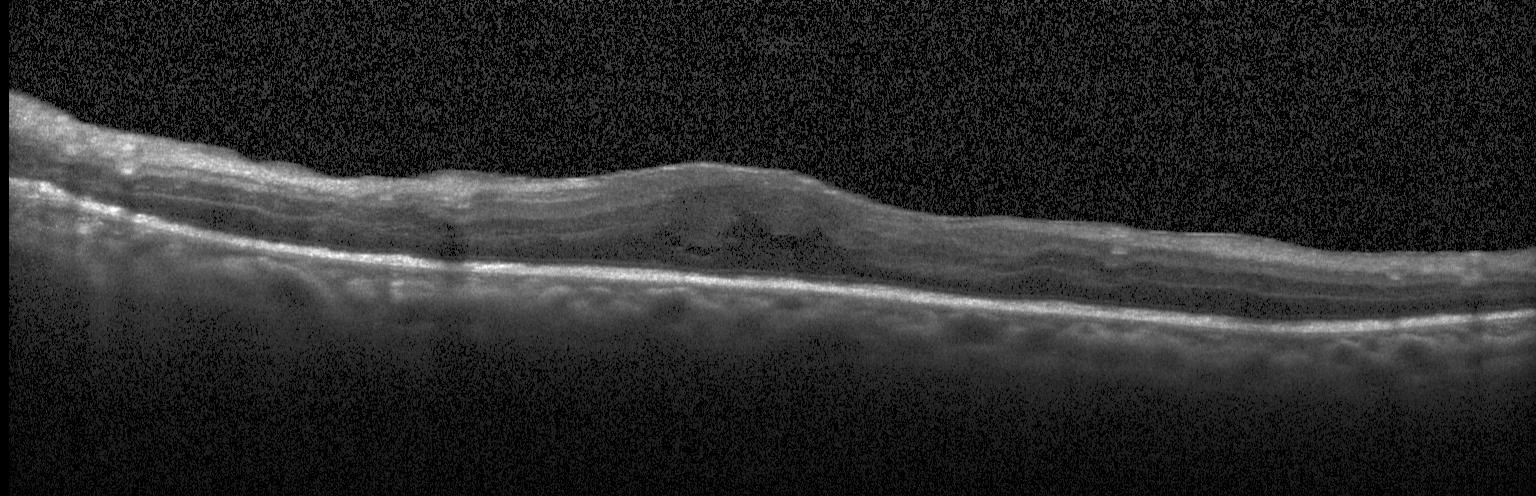
OCT B-scan showing diabetic macular edema (DME).